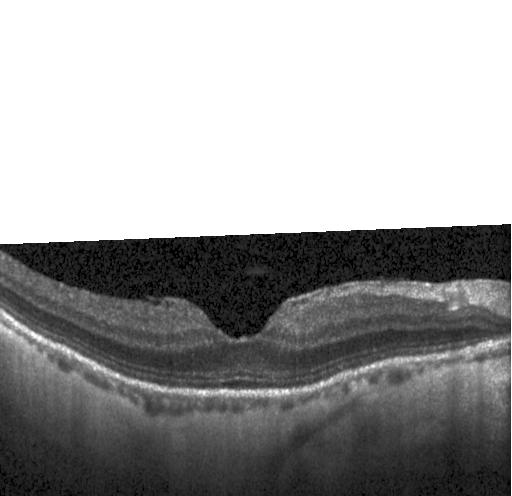 Through the macula. Spectral-domain OCT. Optical coherence tomography B-scan. Diagnosis: neither CNV, DME, nor drusen.